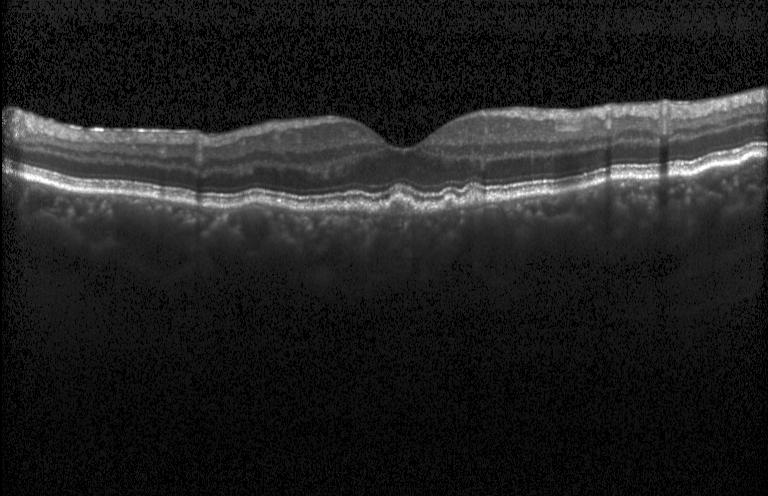
Centered on the fovea; optical coherence tomography B-scan; acquired on a Heidelberg Spectralis.
Dx: drusen.